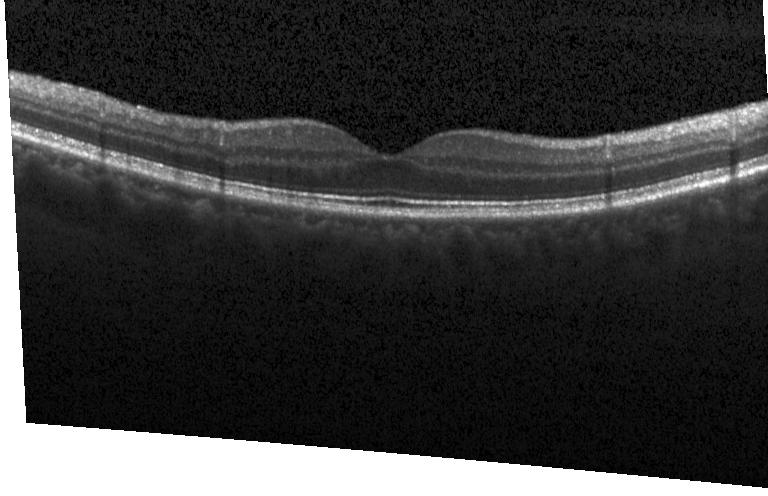 Retinal OCT B-scan · instrument: Heidelberg Spectralis — Diagnosis: neither choroidal neovascularization, diabetic macular edema, nor drusen.